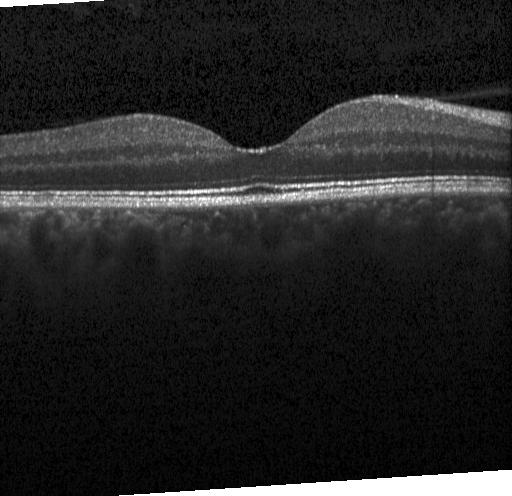 Retinal OCT B-scan · fovea-centered — No evidence of choroidal neovascularization, diabetic macular edema, or drusen.